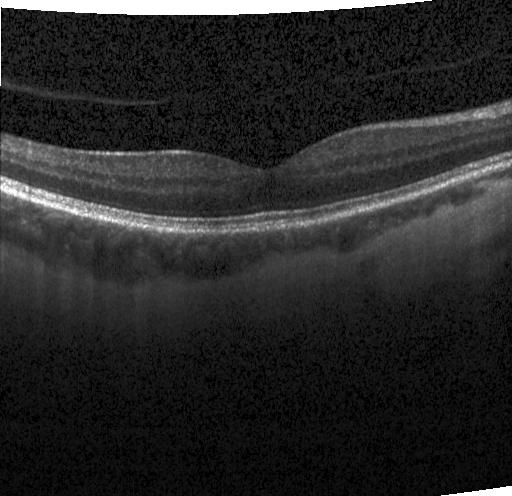
Spectral-domain optical coherence tomography, Heidelberg Spectralis, centered on the fovea, optical coherence tomography scan. OCT finding: no choroidal neovascularization, diabetic macular edema, or drusen.